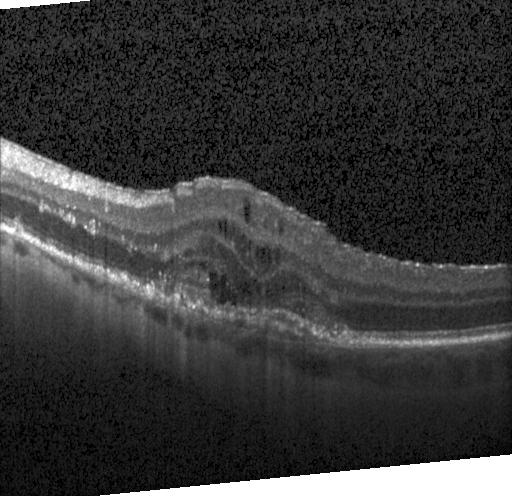

Optical coherence tomography scan — This B-scan demonstrates a choroidal neovascular membrane.